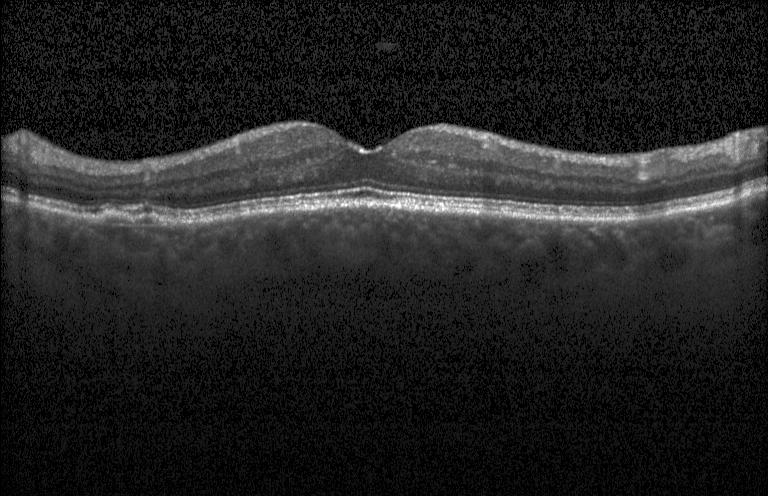

Macular OCT demonstrating CNV.